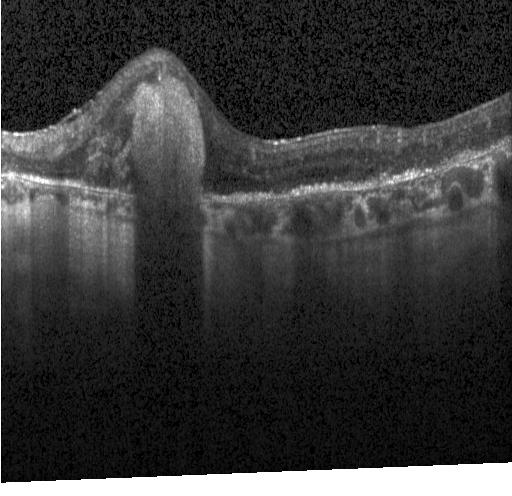 Optical coherence tomography B-scan.
The scan shows a choroidal neovascular membrane.